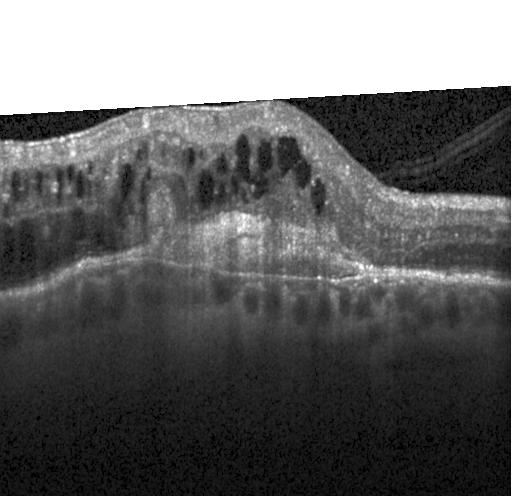 Diagnosis: choroidal neovascularization (CNV).